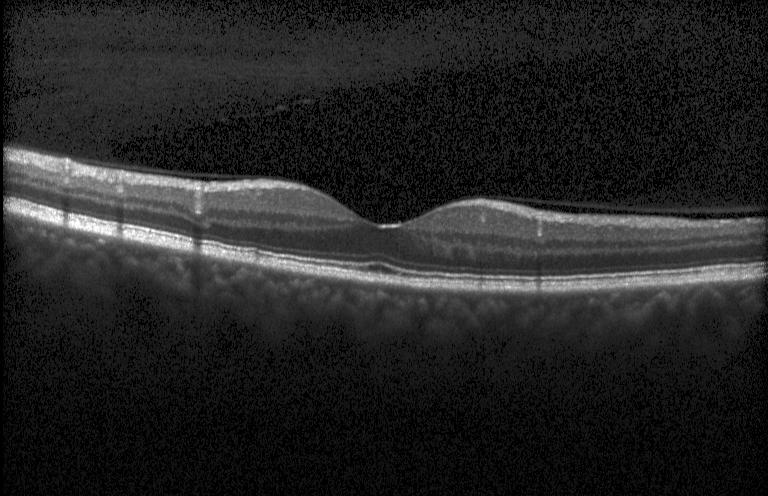
Retinal OCT cross-section — Dx: no choroidal neovascularization, diabetic macular edema, or drusen.